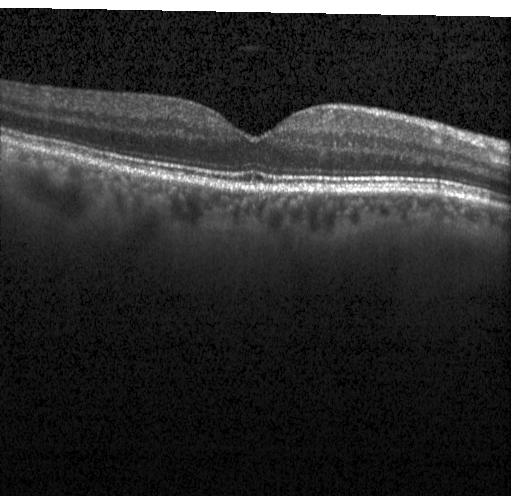

Retinal OCT B-scan. Fovea-centered.
This B-scan demonstrates neither choroidal neovascularization, diabetic macular edema, nor drusen.